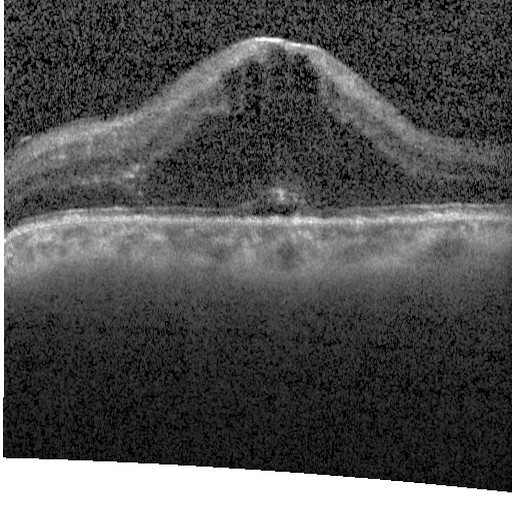
This B-scan demonstrates DME.